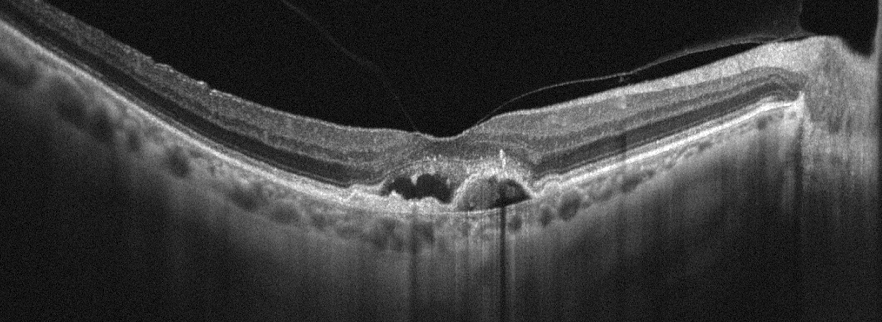

Fovea-centered; OCT line scan; instrument: Optovue Avanti RTVue XR — Finding: AMD.